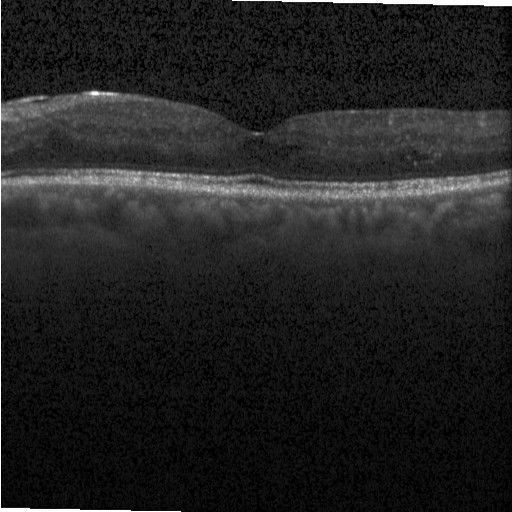 OCT finding: DME.